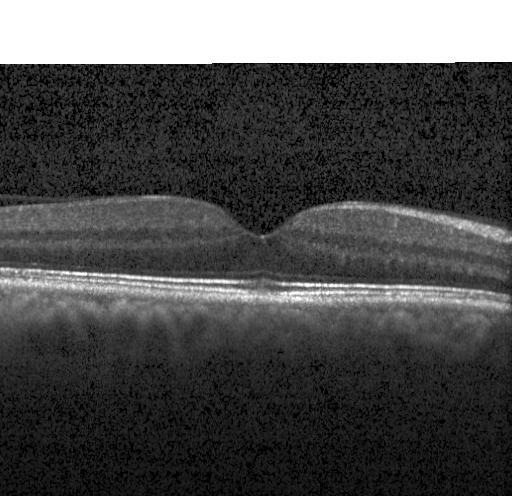

Heidelberg Spectralis OCT system · spectral-domain OCT · horizontal scan through the fovea · retinal OCT B-scan
Diagnosis: no CNV, DME, or drusen.